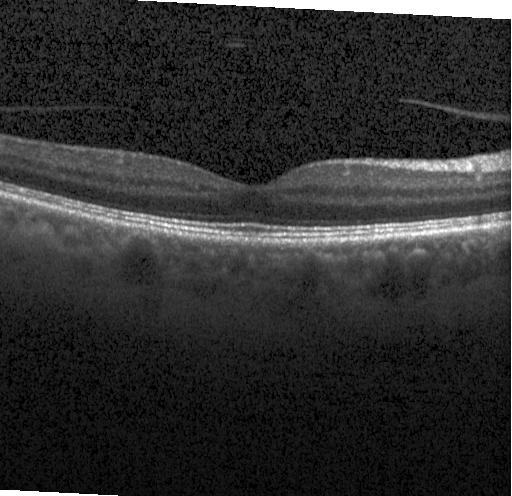
Horizontal scan through the fovea; Heidelberg Spectralis; optical coherence tomography scan; spectral-domain optical coherence tomography.
This B-scan demonstrates no choroidal neovascularization, no diabetic macular edema, and no drusen.